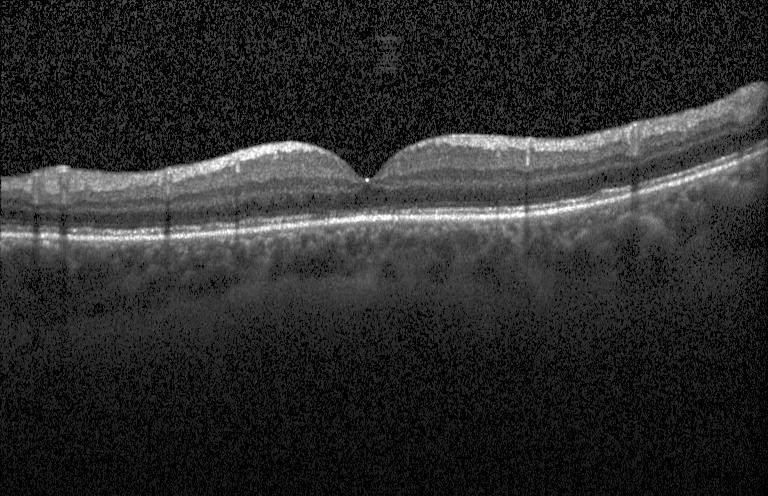
Retinal OCT cross-section. Finding: no choroidal neovascularization, no diabetic macular edema, and no drusen.